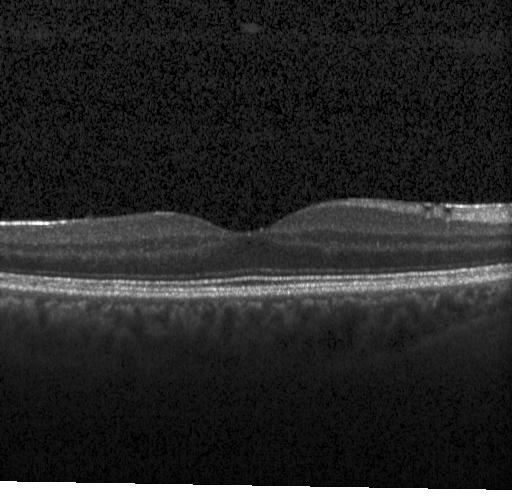 Retinal OCT B-scan, acquired on a Heidelberg Spectralis, SD-OCT
No evidence of choroidal neovascularization, diabetic macular edema, or drusen.